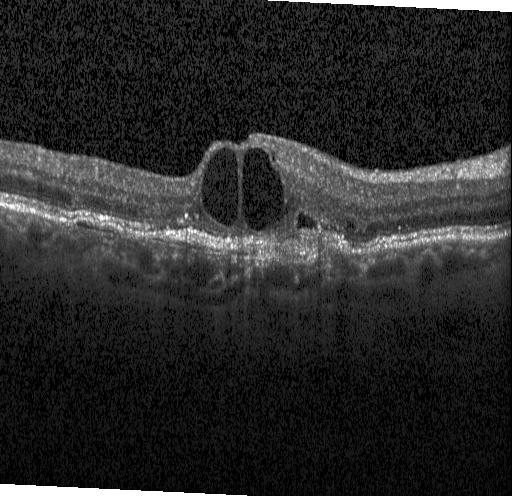
Retinal OCT cross-section. Dx: a choroidal neovascular membrane.